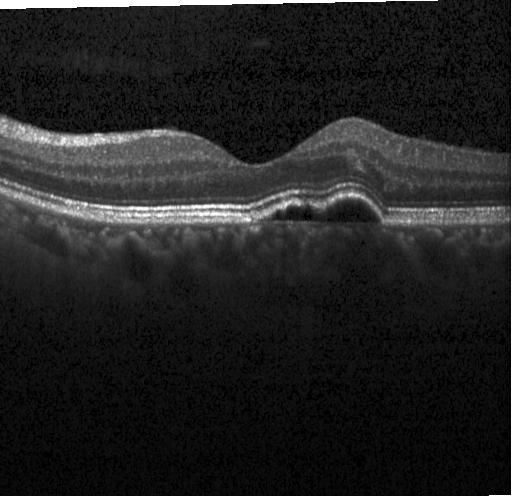 Retinal OCT cross-section. Centered on the fovea. Instrument: Heidelberg Spectralis. Spectral-domain optical coherence tomography — The scan shows a choroidal neovascular membrane.